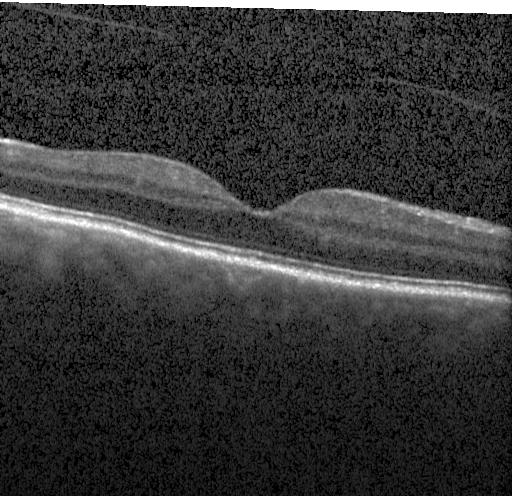
Optical coherence tomography scan; Heidelberg Spectralis.
Diagnosis: no choroidal neovascularization, no diabetic macular edema, and no drusen.